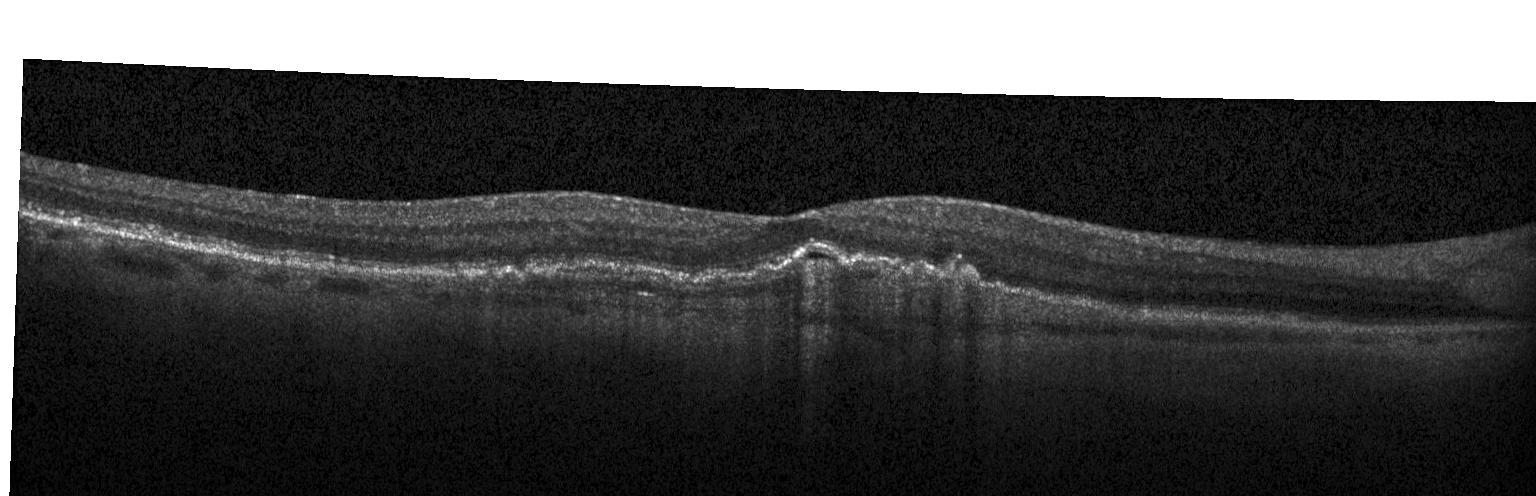

Macular OCT demonstrating choroidal neovascularization.